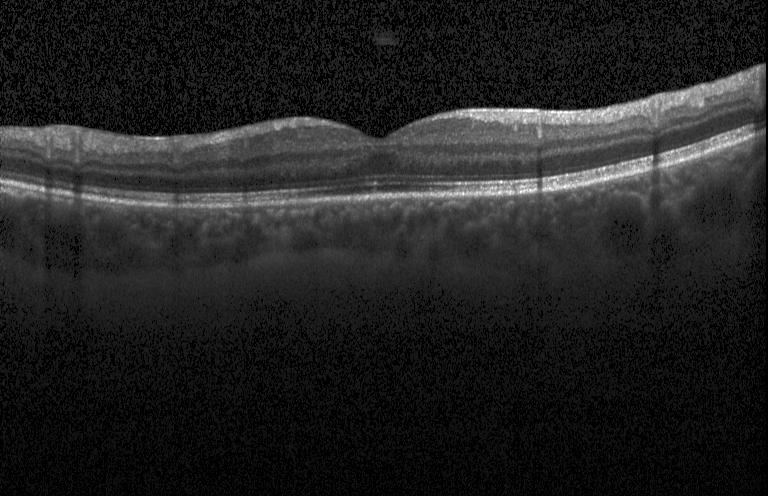

SD-OCT; optical coherence tomography scan; acquired on a Heidelberg Spectralis
Assessment: no choroidal neovascularization, diabetic macular edema, or drusen.